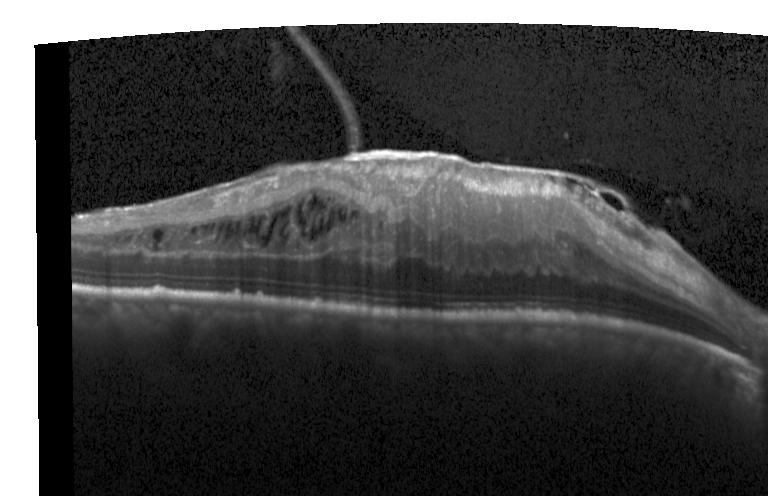

Assessment: diabetic macular edema.